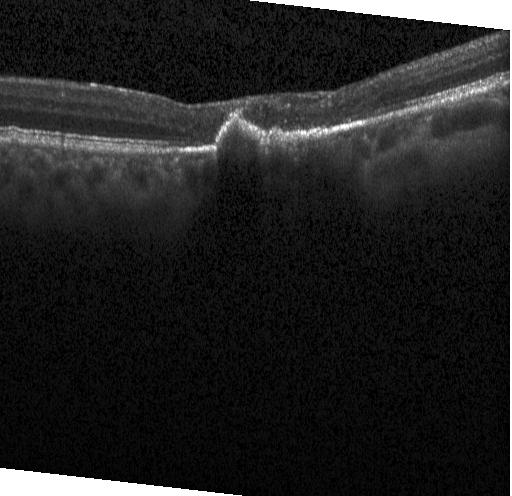

Assessment: CNV.